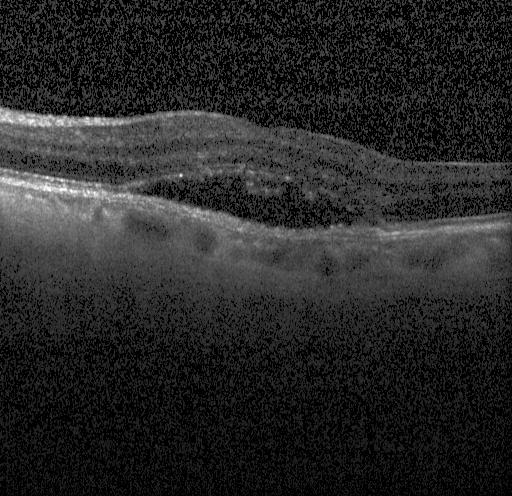

Retinal OCT cross-section showing a choroidal neovascular membrane.